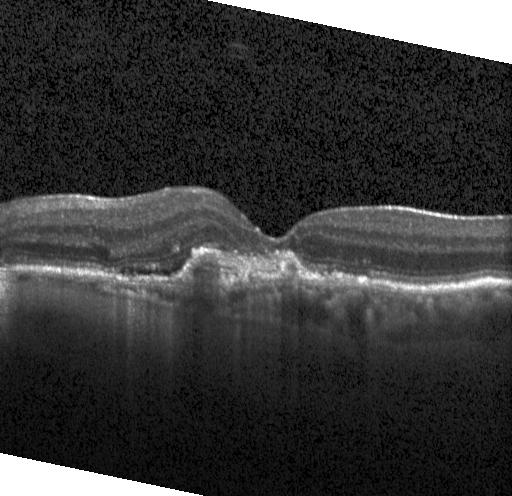 OCT line scan. SD-OCT. Acquired on a Heidelberg Spectralis. Macular scan.
Finding: choroidal neovascularization (CNV).